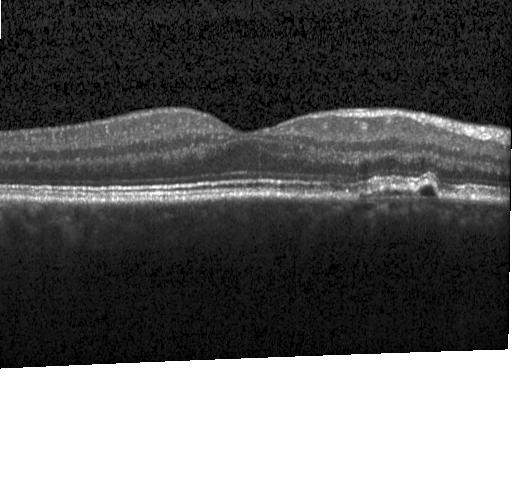

Acquired on a Heidelberg Spectralis. SD-OCT. Fovea-centered. Retinal OCT B-scan
This B-scan demonstrates CNV.